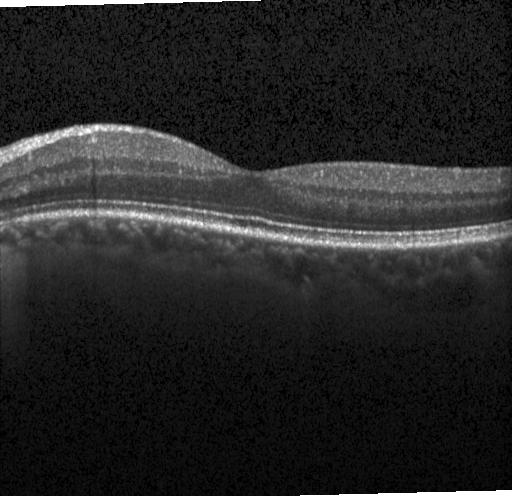 OCT B-scan. Fovea-centered. Spectral-domain optical coherence tomography. Acquired on a Heidelberg Spectralis.
Assessment: no evidence of choroidal neovascularization, diabetic macular edema, or drusen.